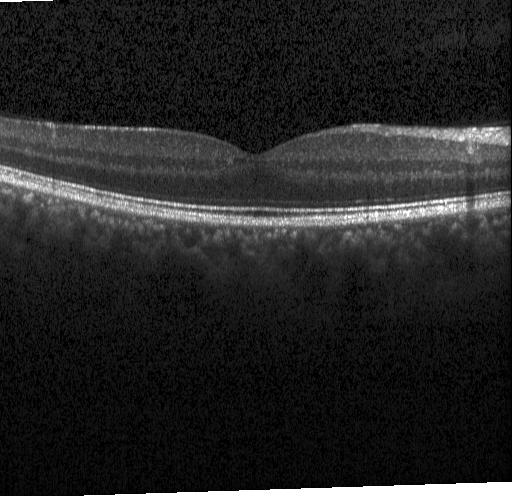
Dx: no evidence of choroidal neovascularization, diabetic macular edema, or drusen.